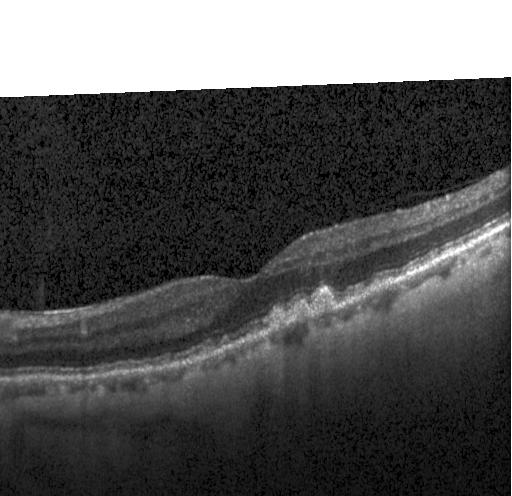 Heidelberg Spectralis · OCT line scan. Dx: drusen.